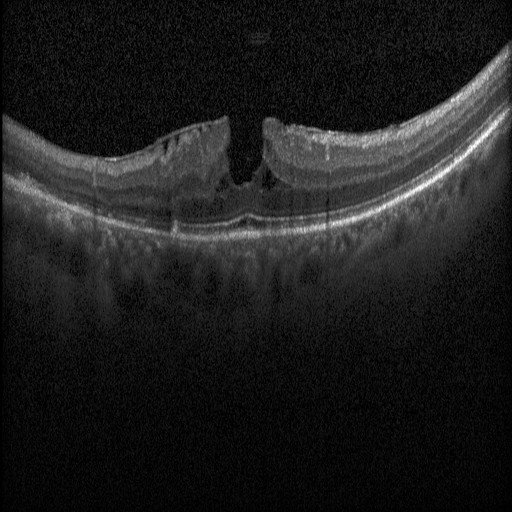

OCT line scan — Impression: diabetic macular edema (DME).